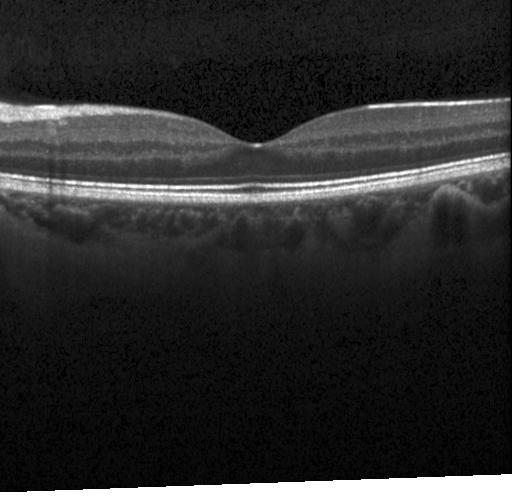
Neither choroidal neovascularization, diabetic macular edema, nor drusen.